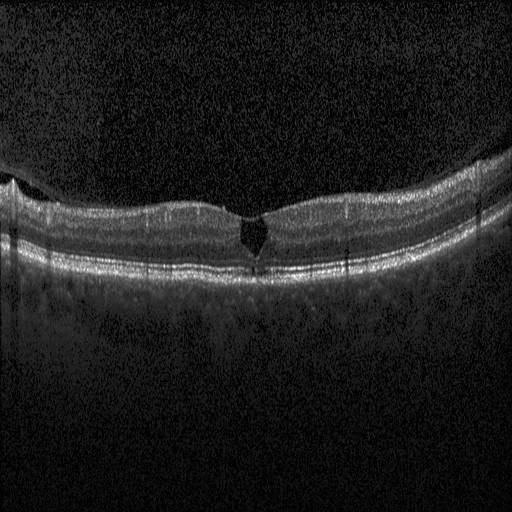

Optical coherence tomography scan. Spectral-domain optical coherence tomography.
Impression: diabetic macular edema (DME).